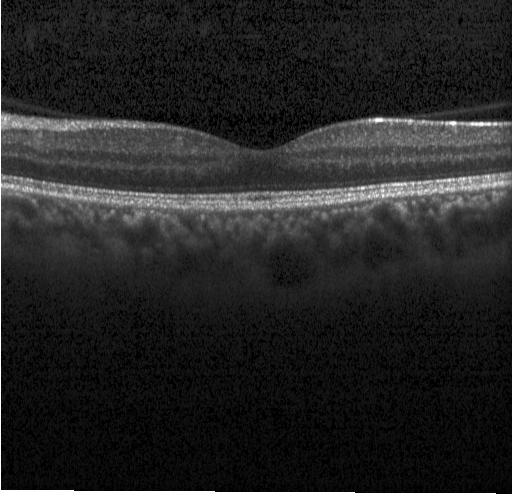 Centered on the fovea. SD-OCT. OCT B-scan
OCT finding: no CNV, DME, or drusen.